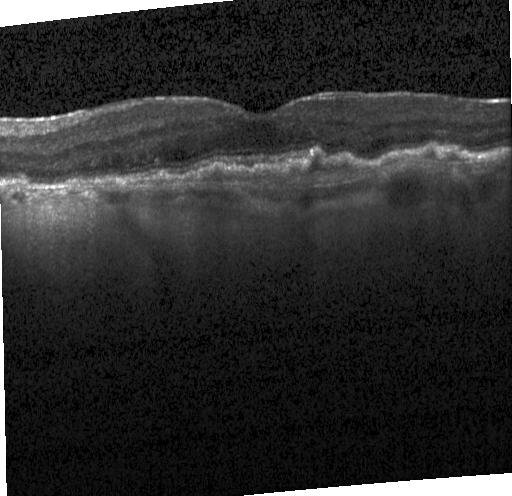

Retinal OCT cross-section showing a choroidal neovascular membrane.